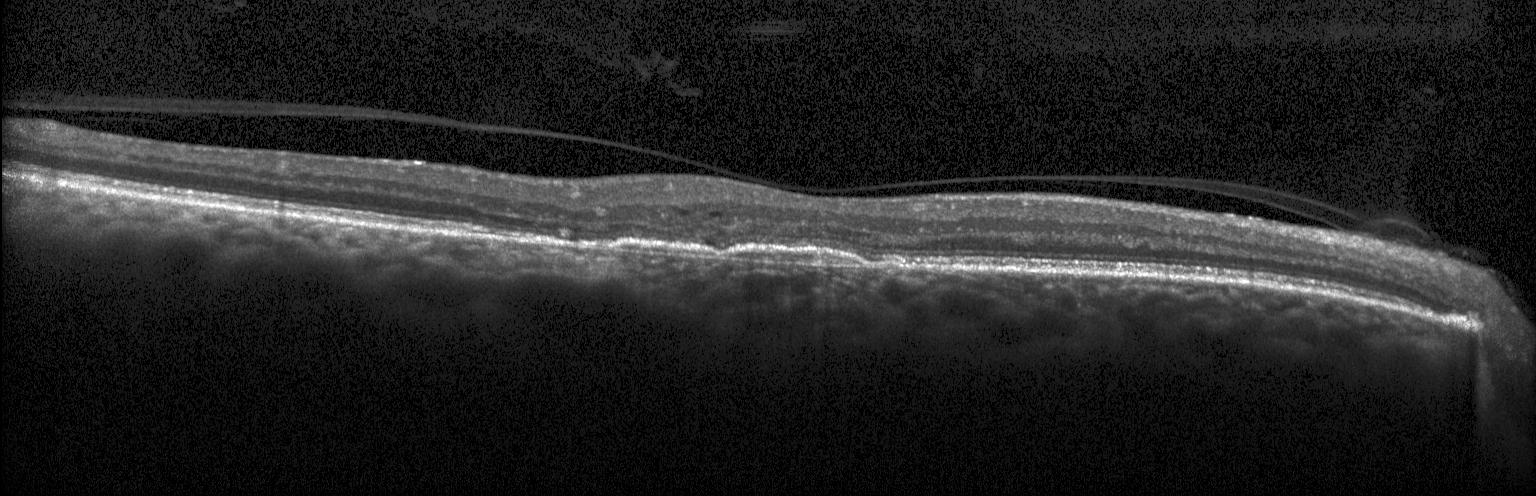
Optical coherence tomography B-scan. Acquired on a Heidelberg Spectralis.
Macular OCT: CNV.